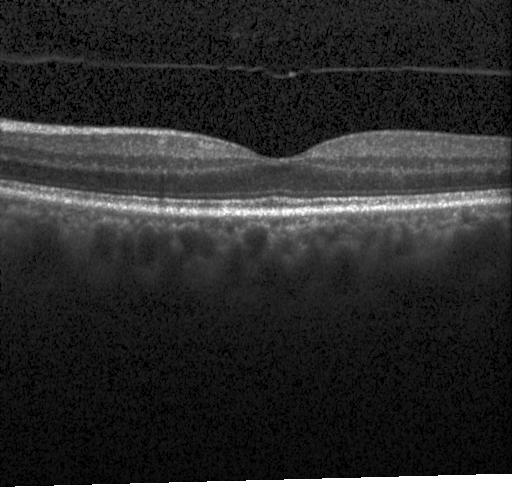 Centered on the fovea. OCT B-scan. SD-OCT. Impression: no CNV, no DME, and no drusen.